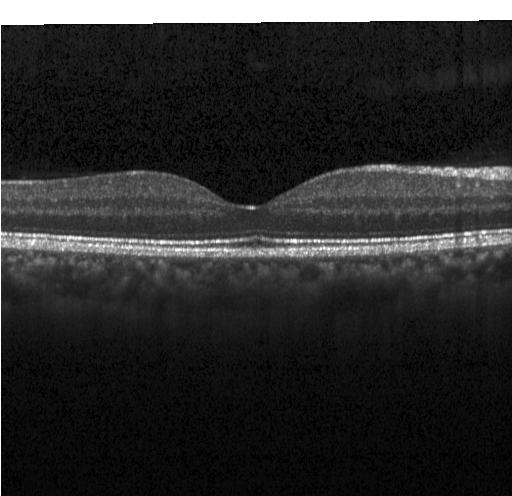

SD-OCT. Instrument: Heidelberg Spectralis. OCT line scan.
The scan shows no choroidal neovascularization, diabetic macular edema, or drusen.